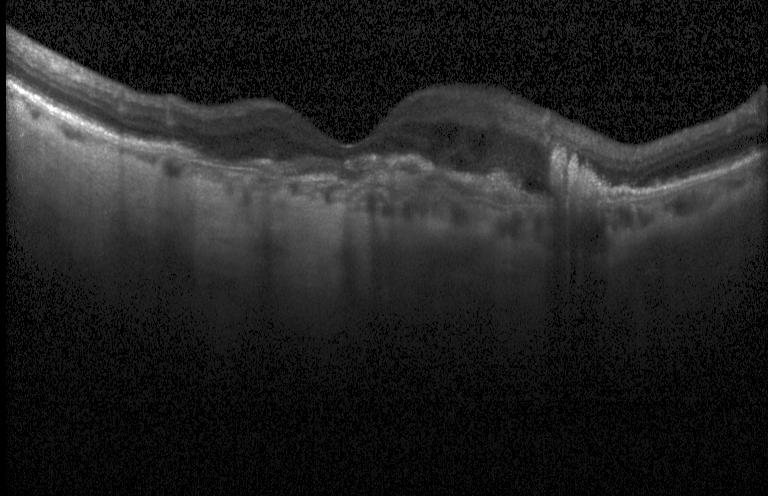

Spectral-domain OCT B-scan: choroidal neovascularization (CNV).